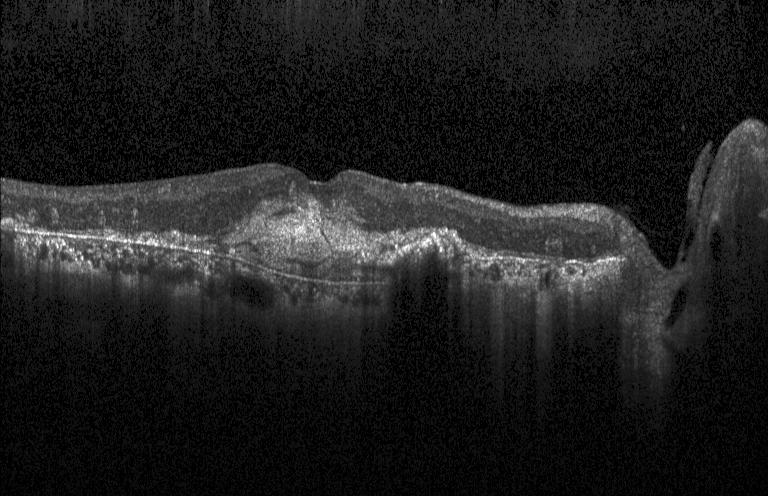
Retinal OCT B-scan. Heidelberg Spectralis OCT system.
Assessment: a choroidal neovascular membrane.